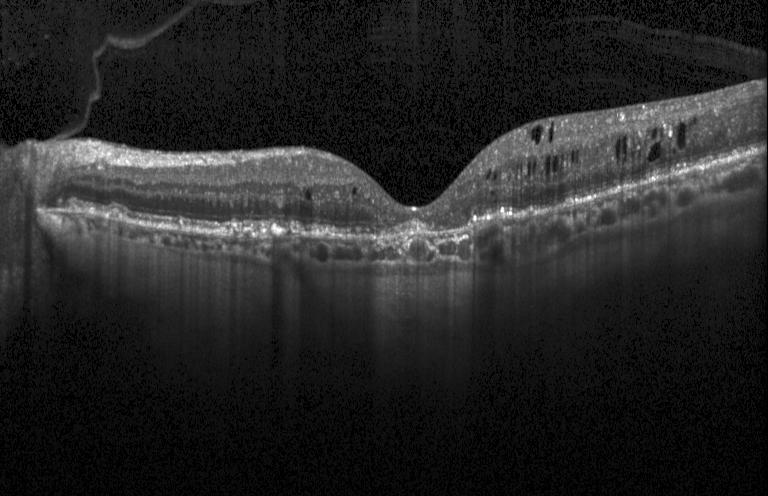

Assessment: a choroidal neovascular membrane.